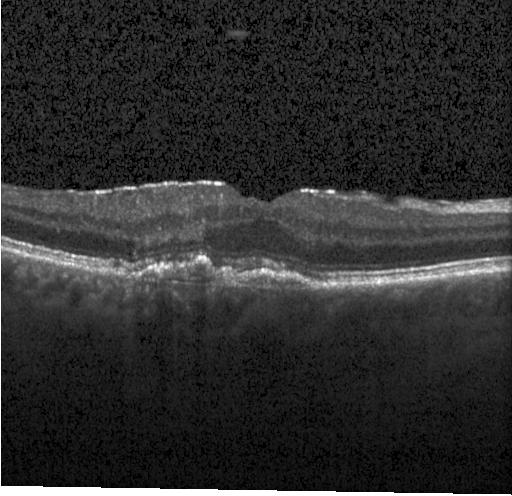 Spectral-domain optical coherence tomography; retinal OCT B-scan; acquired on a Heidelberg Spectralis — Macular OCT: a choroidal neovascular membrane.